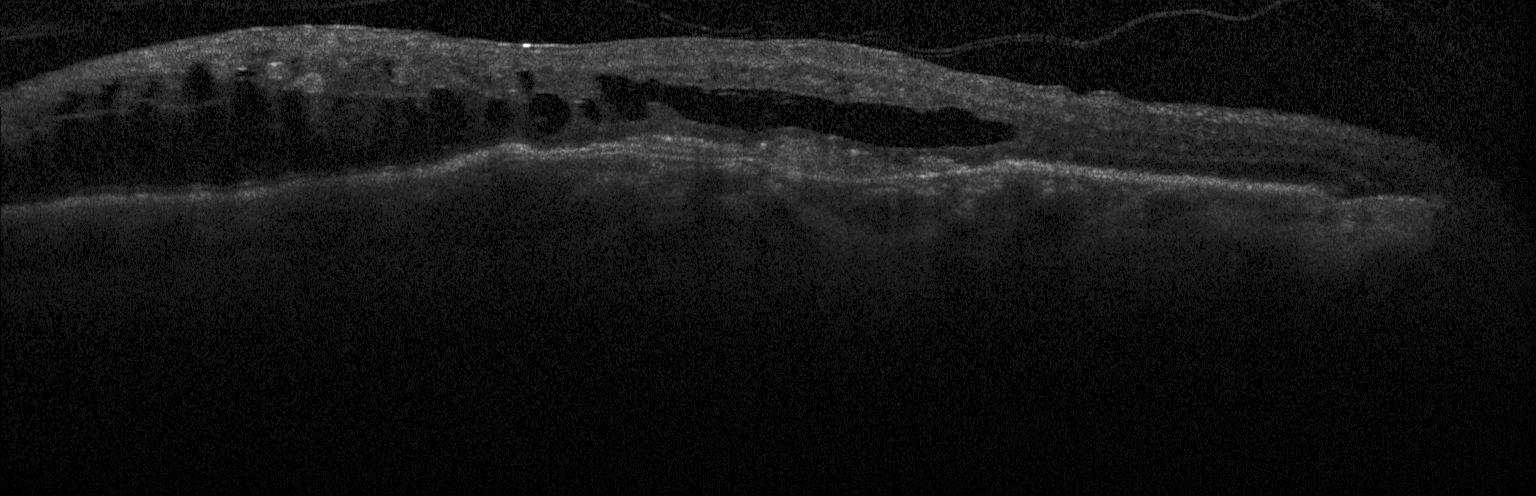

Retinal OCT cross-section showing a choroidal neovascular membrane.